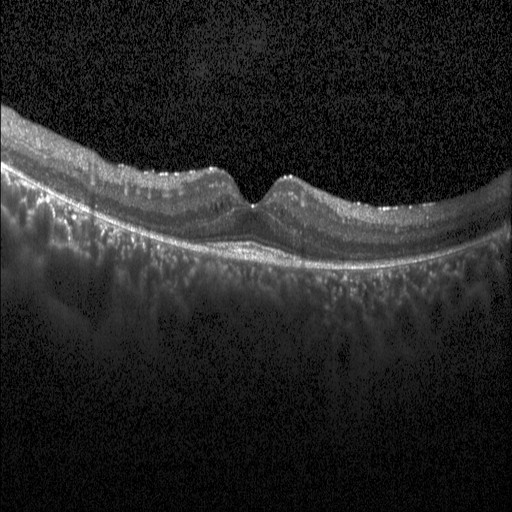
Retinal OCT B-scan · horizontal scan through the fovea. Diagnosis: DME.